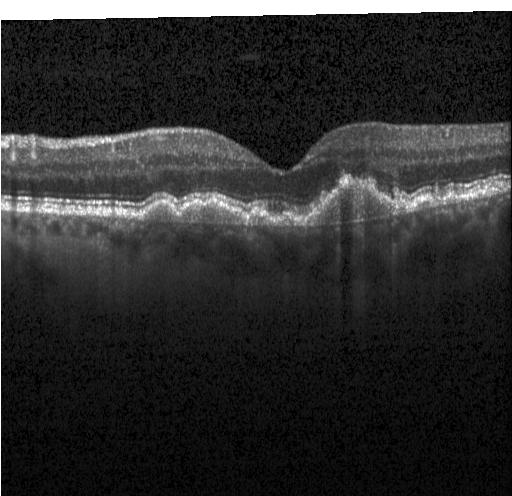 Spectral-domain OCT B-scan: multiple drusen.